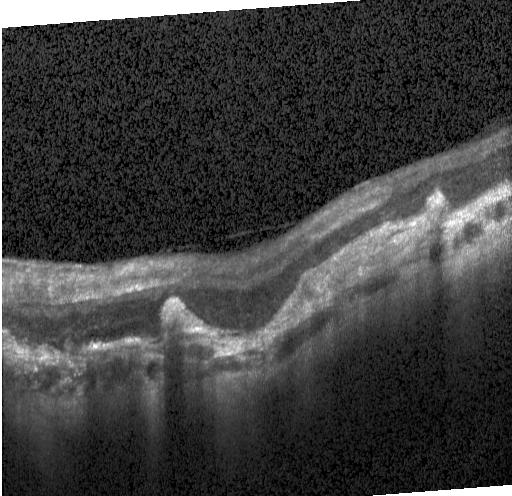

Optical coherence tomography scan · spectral-domain optical coherence tomography · centered on the fovea
Diagnosis: a choroidal neovascular membrane.